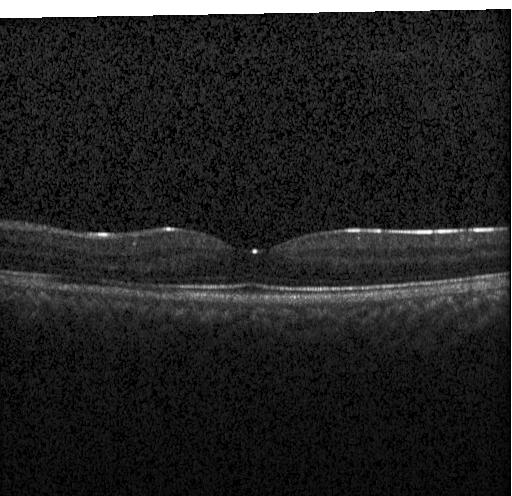

Spectral-domain OCT B-scan: no evidence of choroidal neovascularization, diabetic macular edema, or drusen.